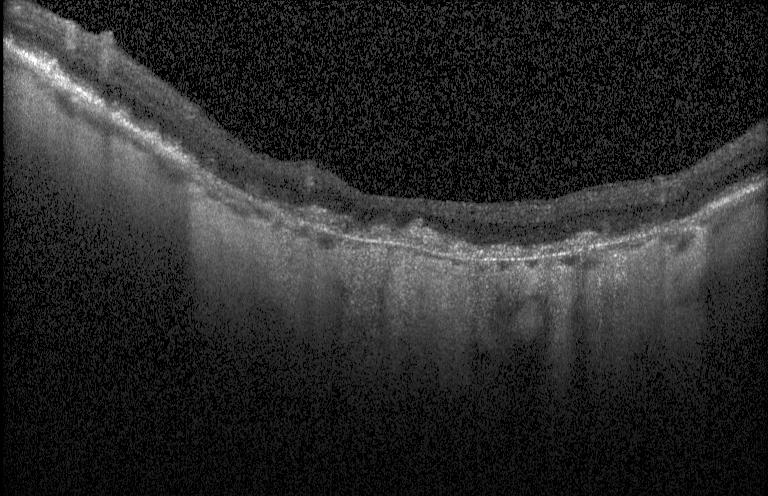
Finding: choroidal neovascularization (CNV).